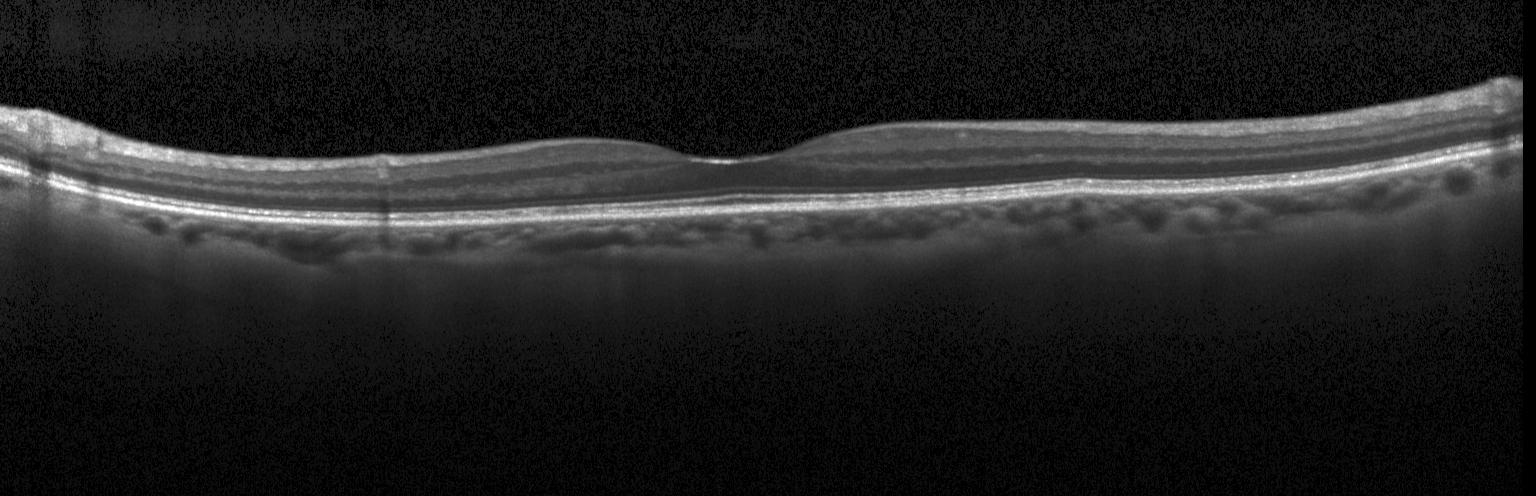
OCT finding: no evidence of choroidal neovascularization, diabetic macular edema, or drusen.